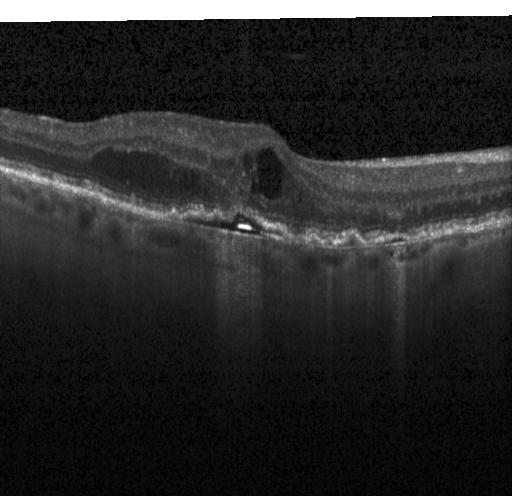 Spectral-domain OCT · optical coherence tomography B-scan
Finding: CNV.